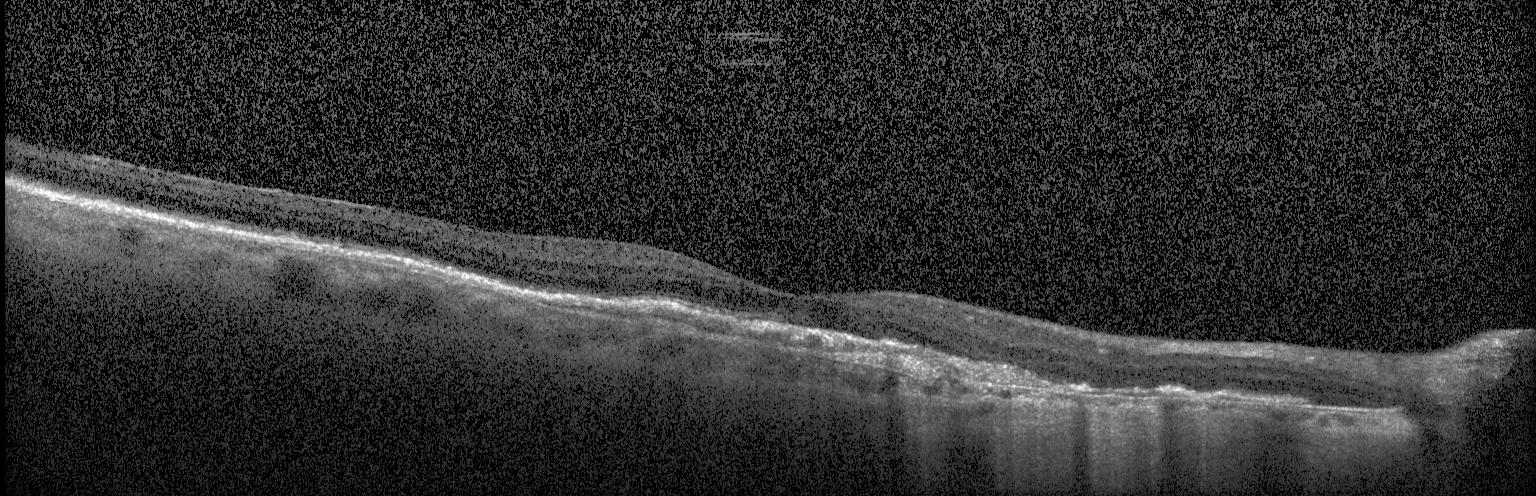

OCT finding: CNV.